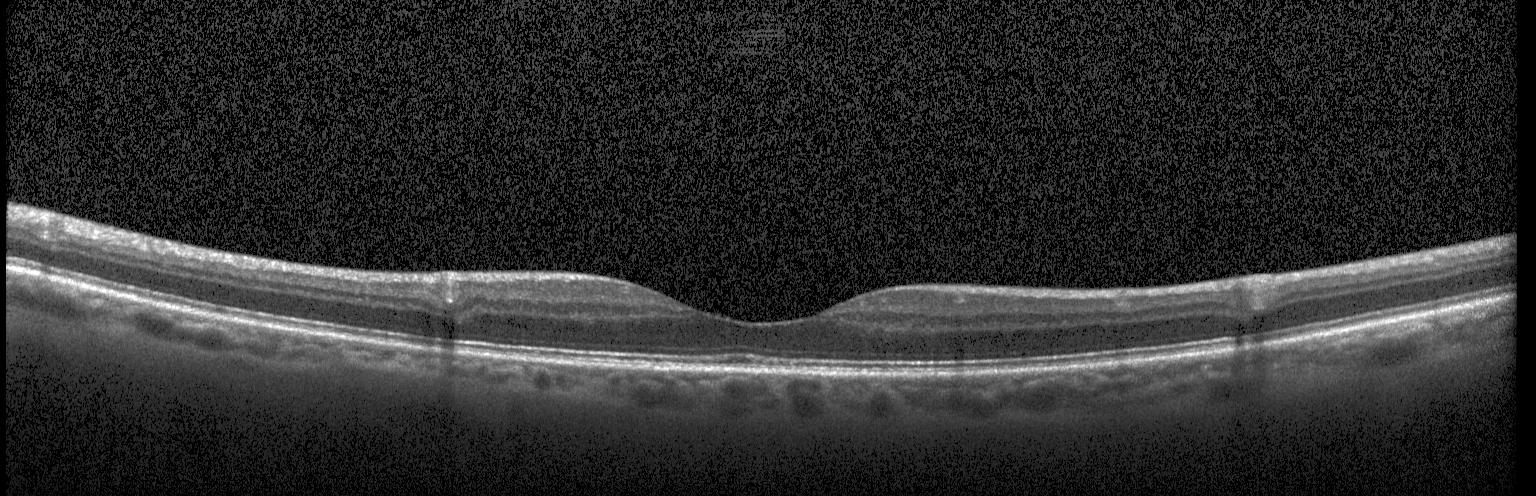

This B-scan demonstrates no CNV, no DME, and no drusen.